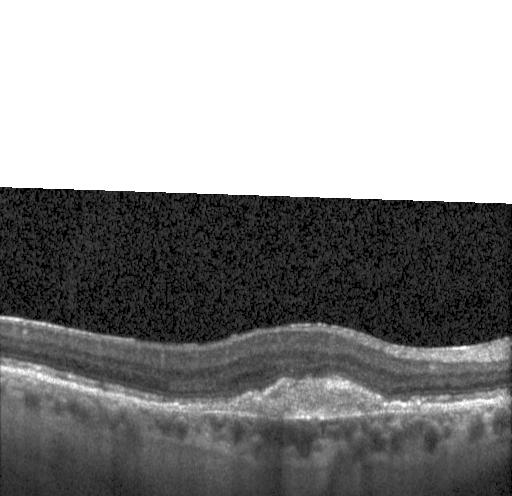

OCT B-scan; SD-OCT.
Macular OCT: CNV.